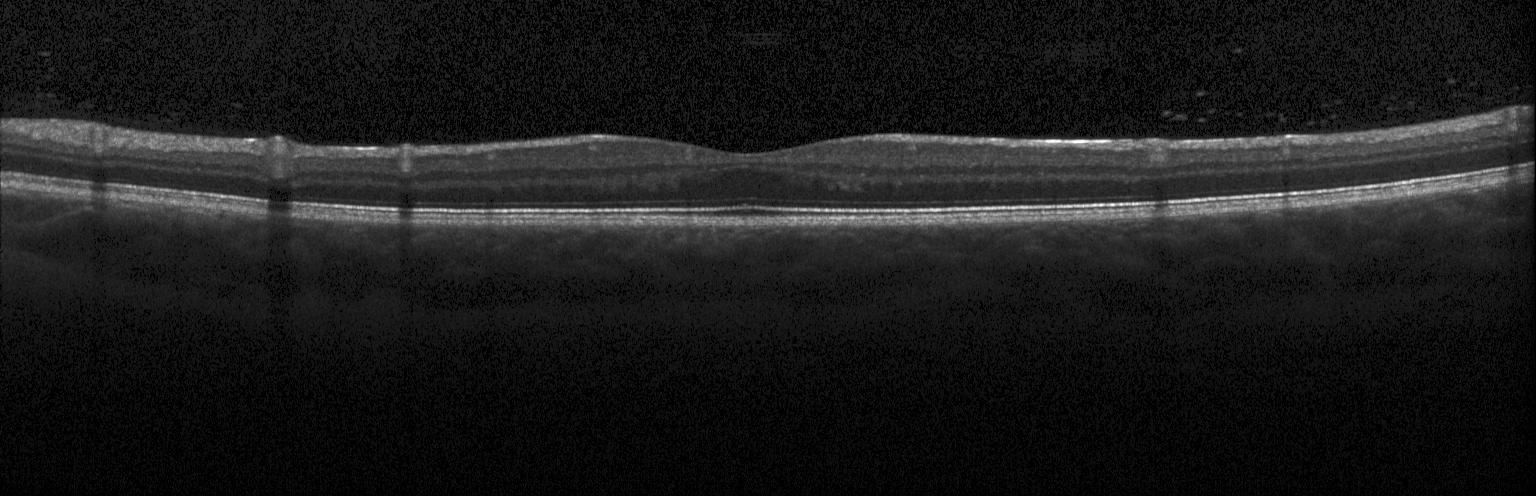
Spectral-domain OCT B-scan: neither CNV, DME, nor drusen.